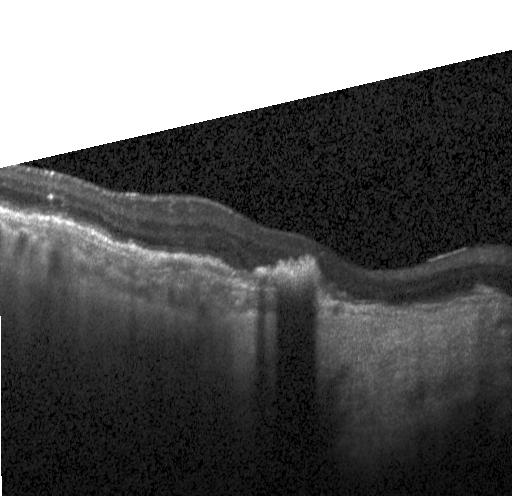
Optical coherence tomography B-scan, spectral-domain OCT, centered on the fovea, acquired on a Heidelberg Spectralis — OCT finding: choroidal neovascularization.